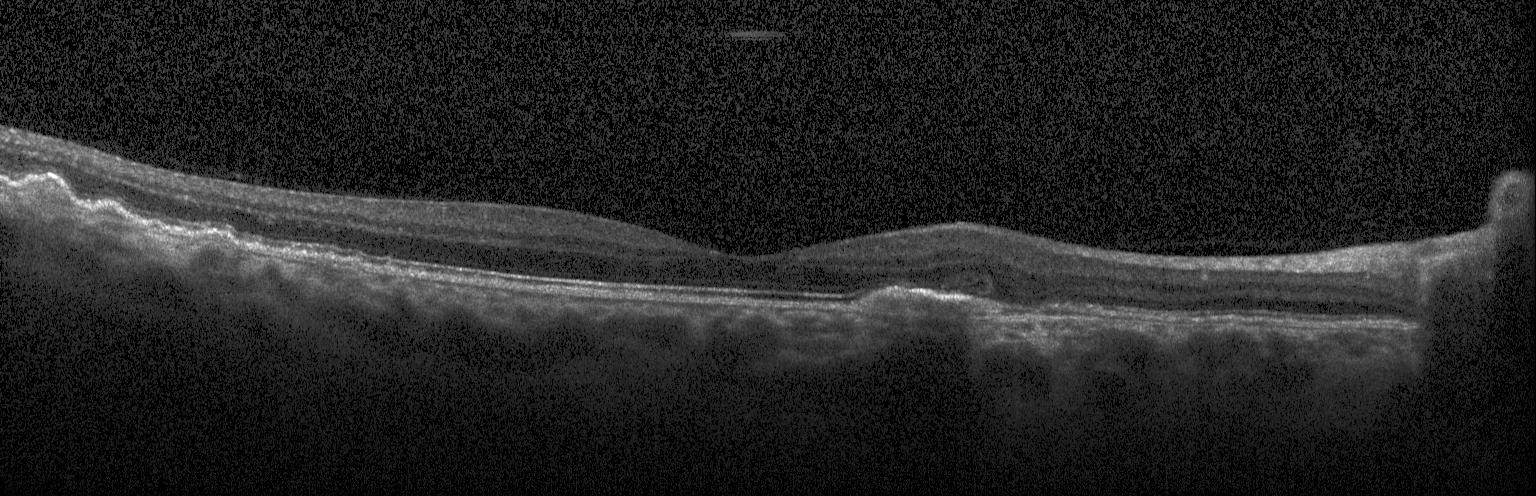
Assessment: choroidal neovascularization (CNV).